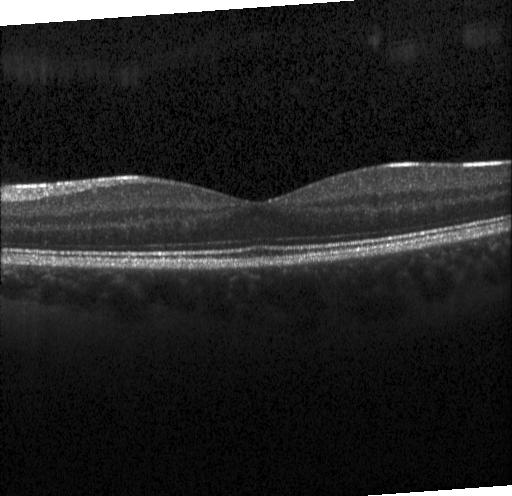 Retinal OCT B-scan — Finding: no choroidal neovascularization, no diabetic macular edema, and no drusen.